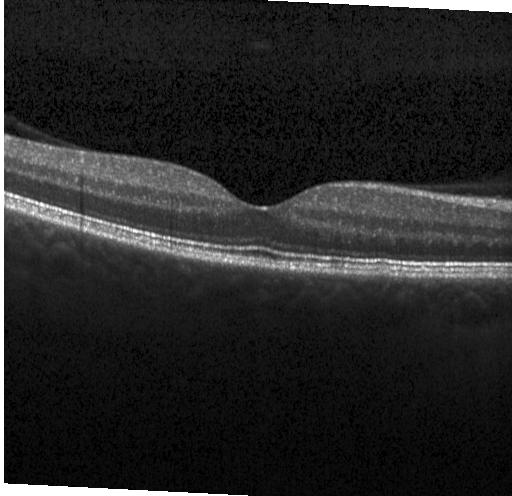
Horizontal scan through the fovea; retinal OCT B-scan.
Dx: neither choroidal neovascularization, diabetic macular edema, nor drusen.